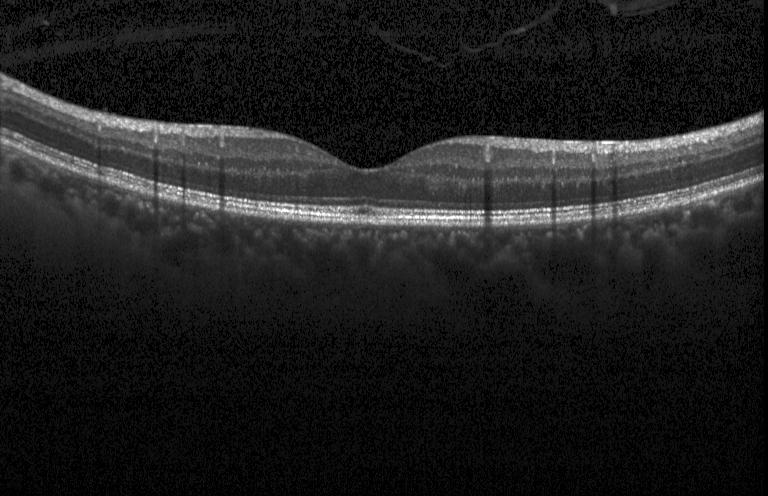

Finding: no choroidal neovascularization, no diabetic macular edema, and no drusen.